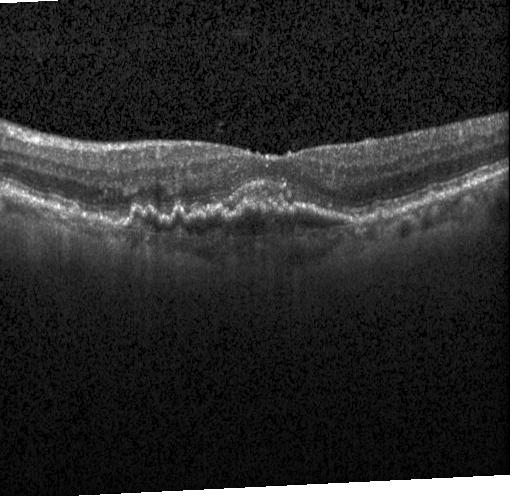
Fovea-centered · Heidelberg Spectralis OCT system · optical coherence tomography B-scan · SD-OCT — Diagnosis: a choroidal neovascular membrane.